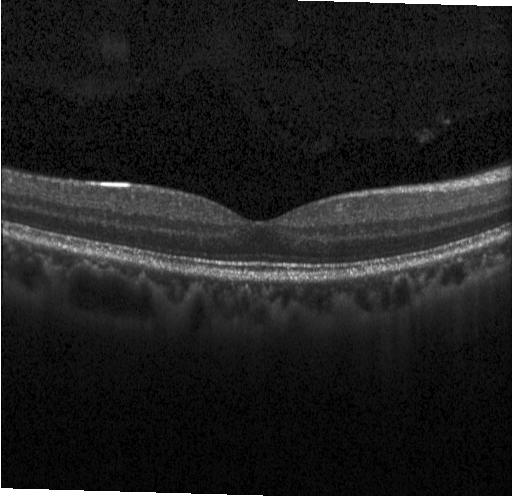

OCT scan showing no evidence of choroidal neovascularization, diabetic macular edema, or drusen.